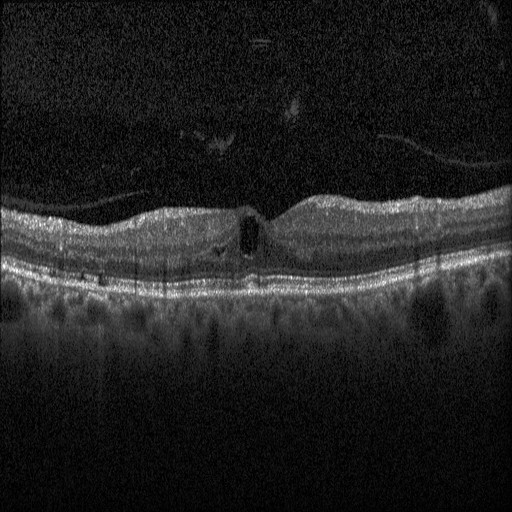

Heidelberg Spectralis · OCT line scan — Assessment: diabetic macular edema.